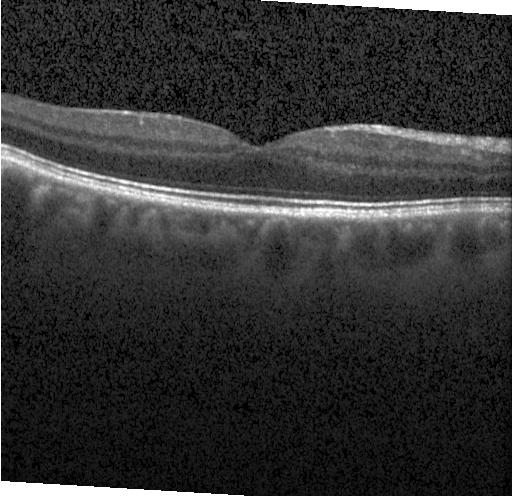
Fovea-centered. SD-OCT. Retinal OCT B-scan
Diagnosis: no evidence of choroidal neovascularization, diabetic macular edema, or drusen.